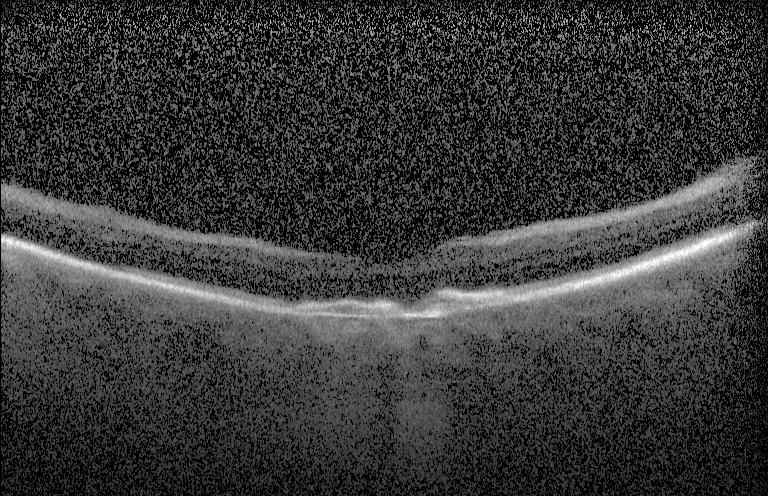 Dx: choroidal neovascularization.